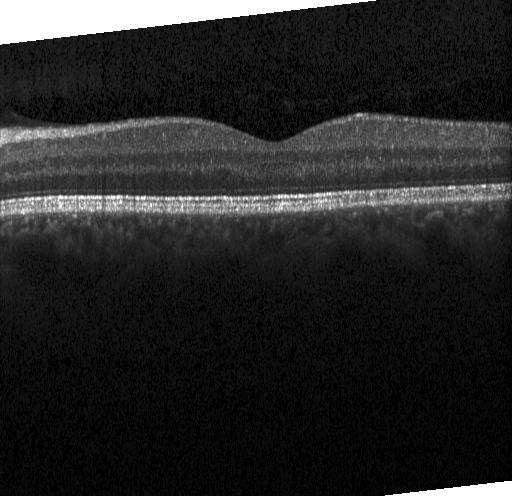

Dx: no evidence of choroidal neovascularization, diabetic macular edema, or drusen.